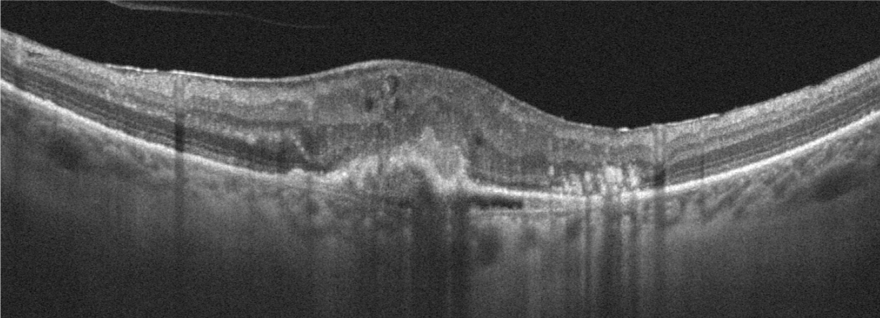

Impression: age-related macular degeneration (AMD).